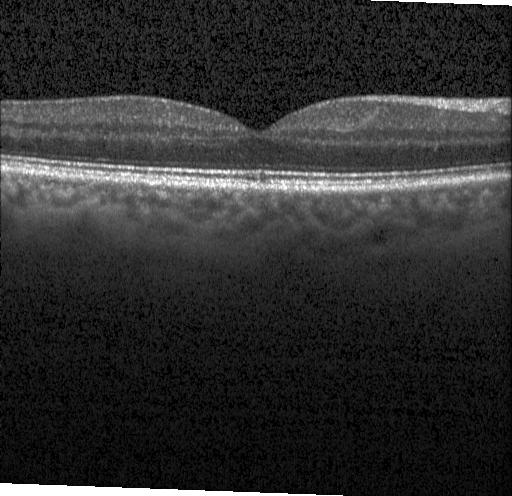 Retinal OCT cross-section, centered on the fovea, Heidelberg Spectralis
Dx: neither choroidal neovascularization, diabetic macular edema, nor drusen.